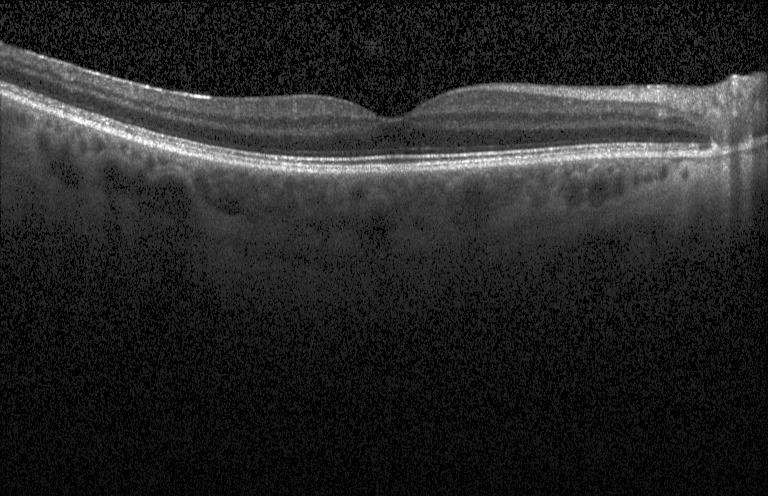
Spectral-domain OCT B-scan: no evidence of CNV, DME, or drusen.